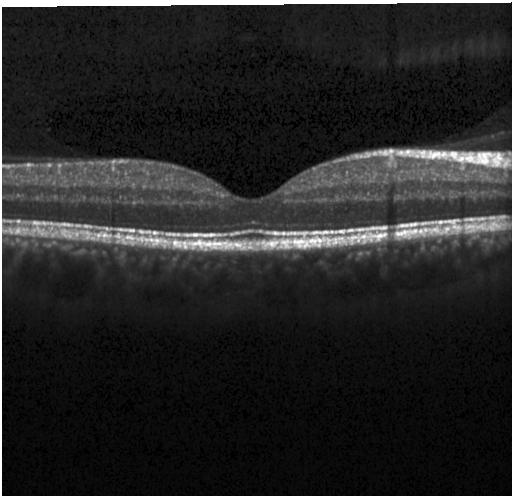
Assessment: no evidence of CNV, DME, or drusen.